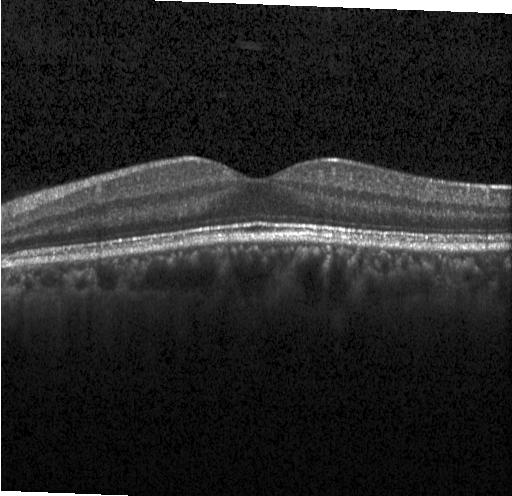
Through the macula, OCT line scan. Diagnosis: no evidence of choroidal neovascularization, diabetic macular edema, or drusen.